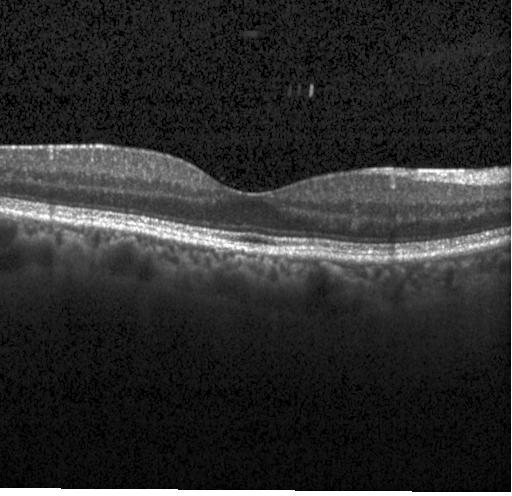 OCT B-scan showing neither choroidal neovascularization, diabetic macular edema, nor drusen.